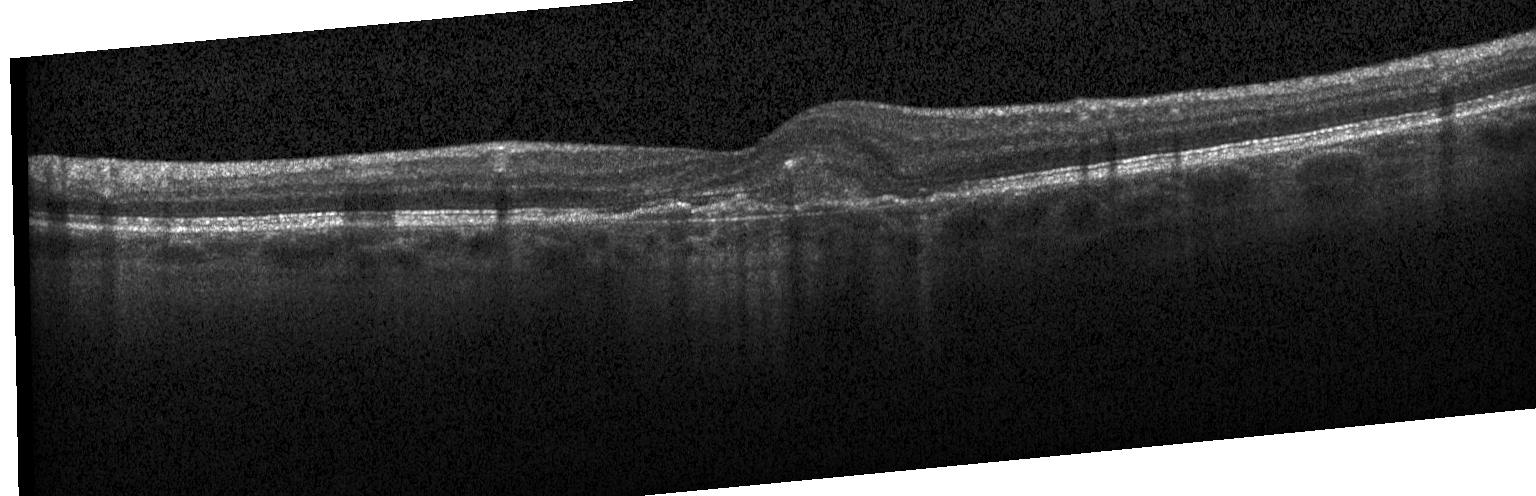 Spectral-domain OCT B-scan: CNV.